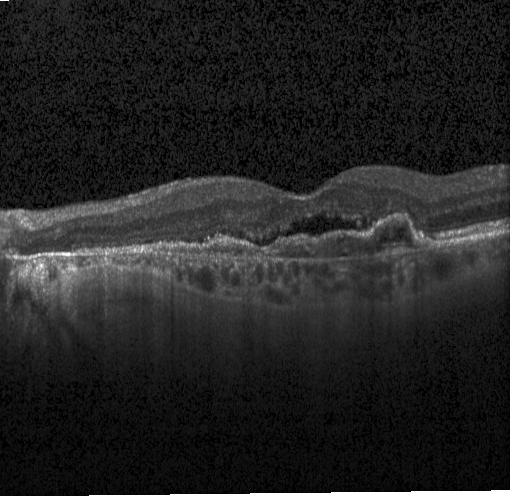

Macular OCT: a choroidal neovascular membrane.